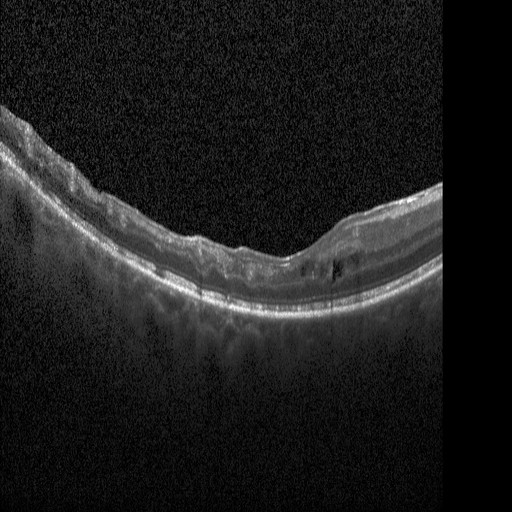
Finding: diabetic macular edema.